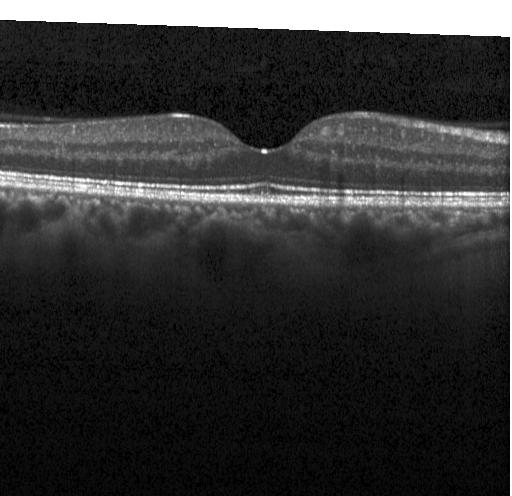

Optical coherence tomography scan — Assessment: neither CNV, DME, nor drusen.